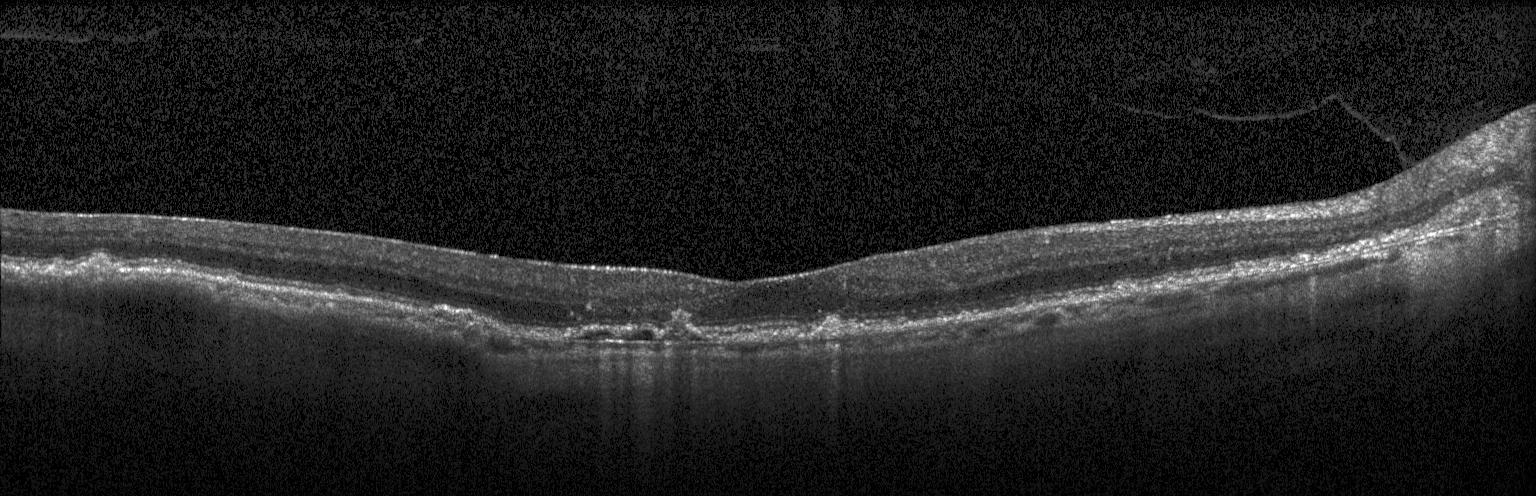

Horizontal scan through the fovea, spectral-domain OCT, instrument: Heidelberg Spectralis, OCT line scan.
This B-scan demonstrates a choroidal neovascular membrane.